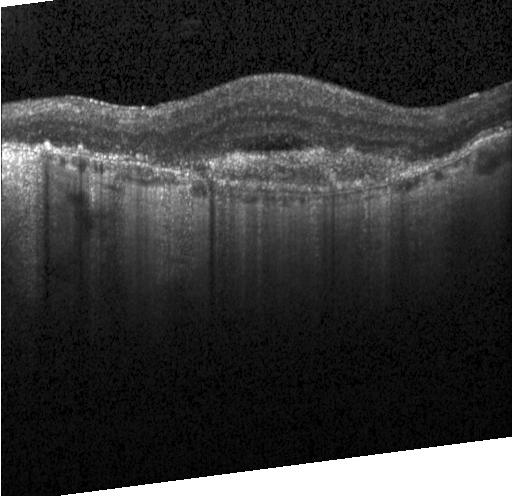 Centered on the fovea. Acquired on a Heidelberg Spectralis. Spectral-domain optical coherence tomography. Optical coherence tomography B-scan — This B-scan demonstrates choroidal neovascularization.